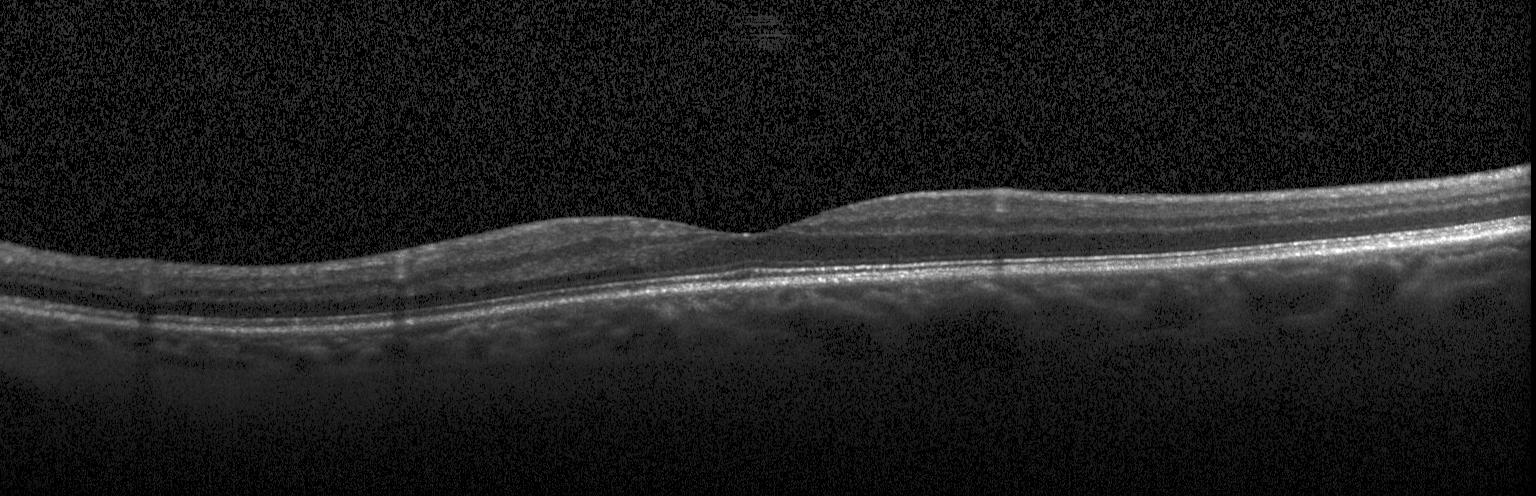
Optical coherence tomography scan.
This B-scan demonstrates no choroidal neovascularization, diabetic macular edema, or drusen.